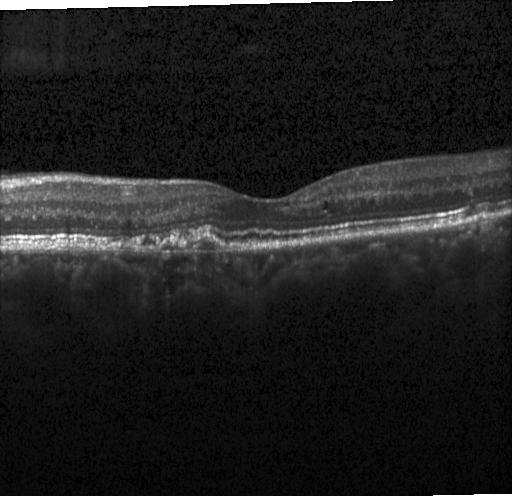
Assessment: CNV.